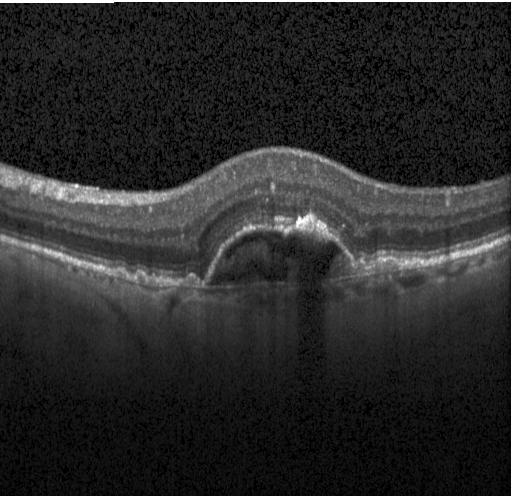 Diagnosis: a choroidal neovascular membrane.